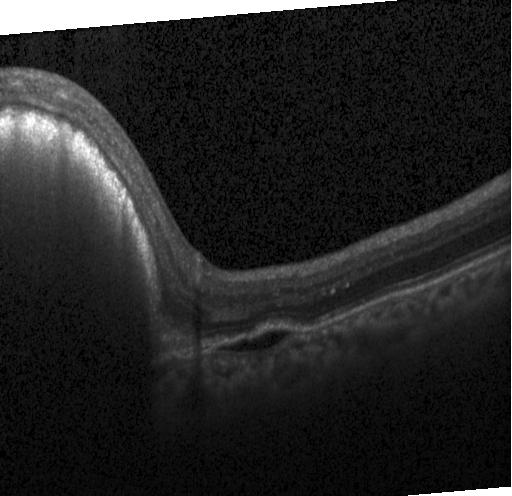

Finding: CNV.